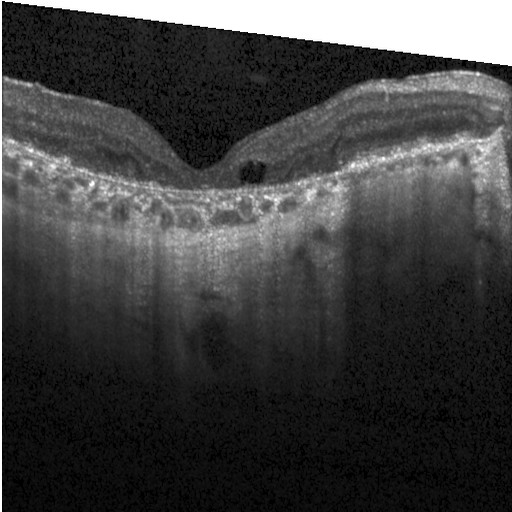 Finding: DME.